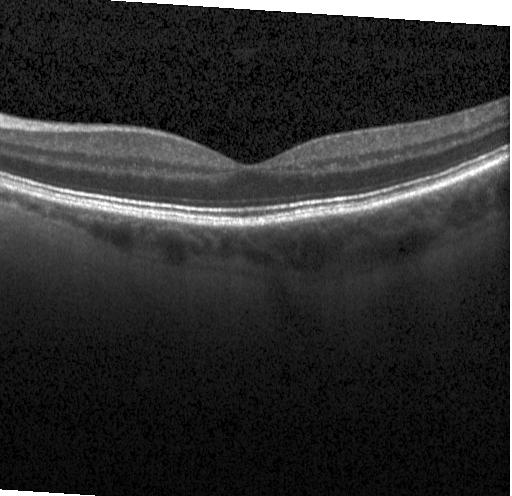 OCT line scan — Diagnosis: no CNV, no DME, and no drusen.